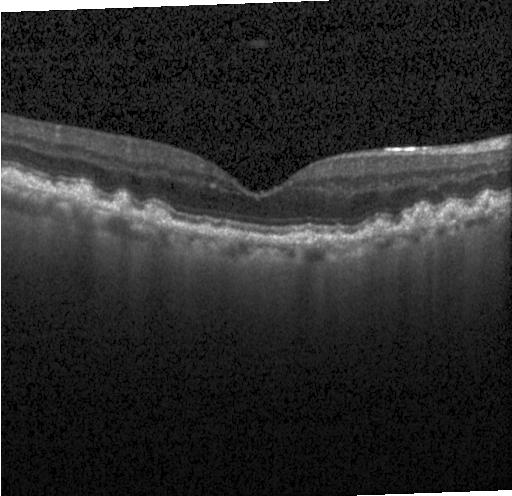

Acquired on a Heidelberg Spectralis · horizontal scan through the fovea · OCT B-scan — Diagnosis: sub-RPE drusenoid deposits.